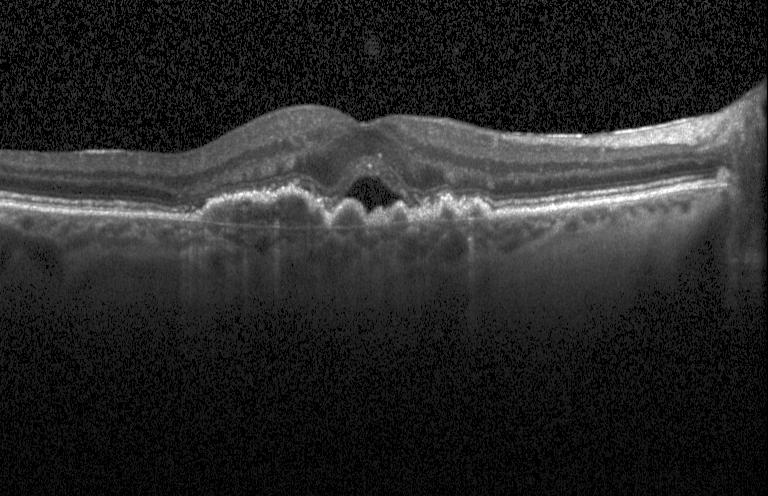 Macular scan; optical coherence tomography scan; SD-OCT.
Assessment: a choroidal neovascular membrane.